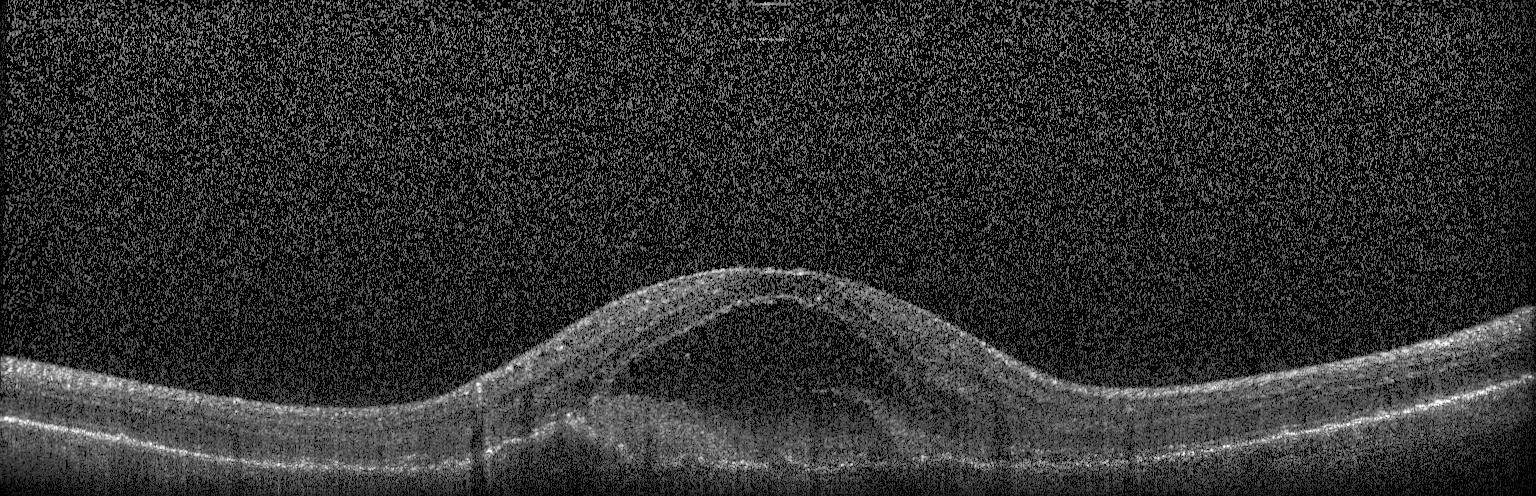
OCT B-scan — Dx: choroidal neovascularization.